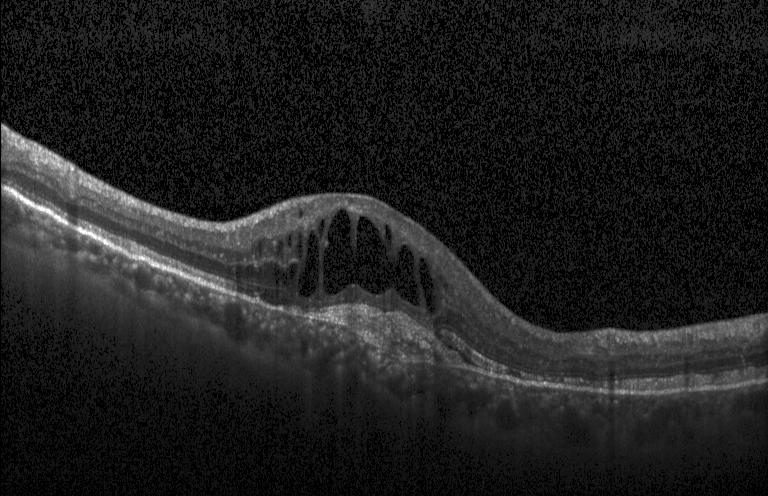

OCT finding: CNV.